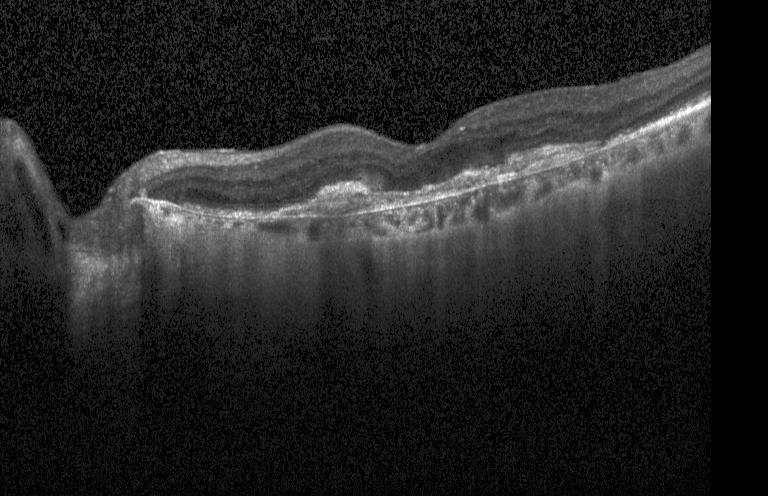
Retinal OCT B-scan · Heidelberg Spectralis OCT system · spectral-domain OCT
OCT finding: choroidal neovascularization (CNV).